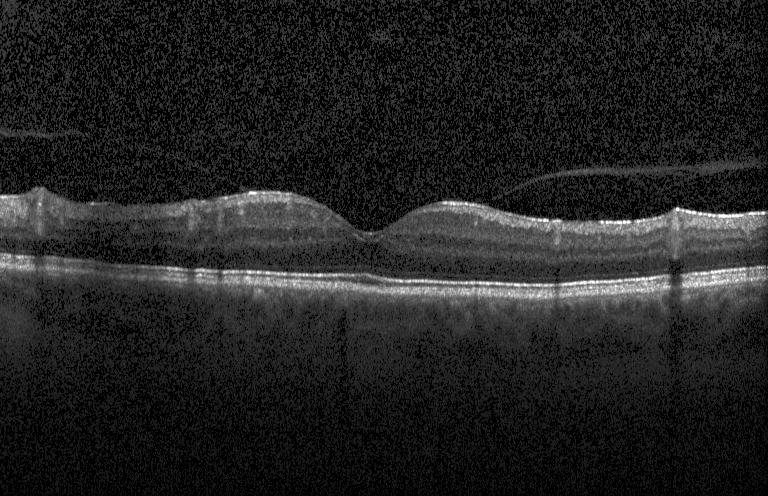

Diagnosis: neither CNV, DME, nor drusen.